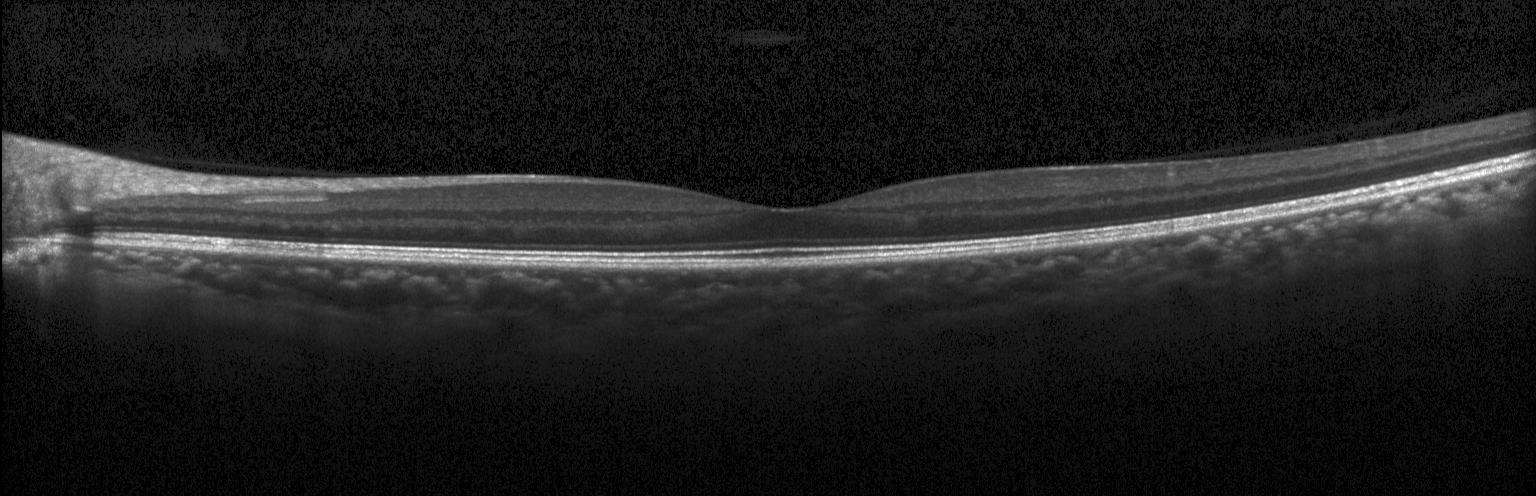 Impression: no evidence of choroidal neovascularization, diabetic macular edema, or drusen.